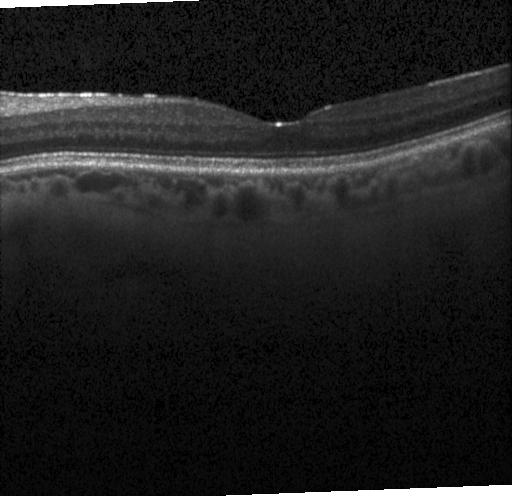
Heidelberg Spectralis, optical coherence tomography B-scan, spectral-domain optical coherence tomography, macular scan
No evidence of CNV, DME, or drusen.